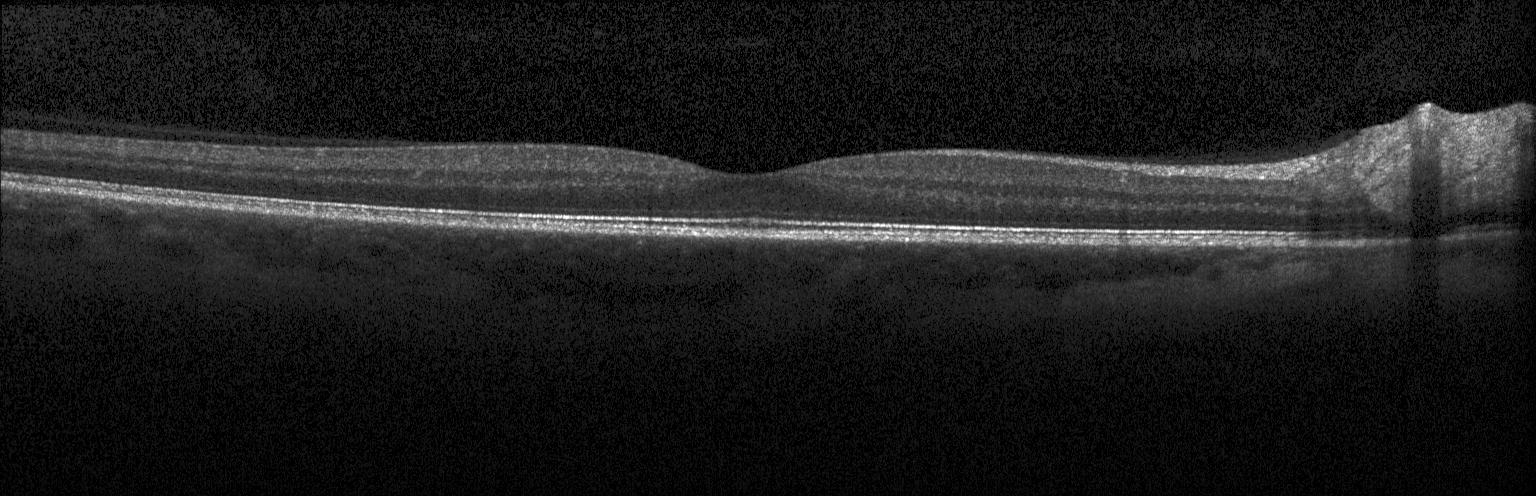 OCT finding: no evidence of choroidal neovascularization, diabetic macular edema, or drusen.